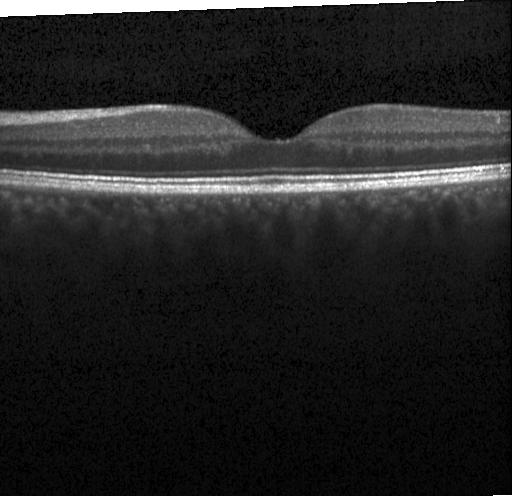

OCT line scan.
Macular OCT: no choroidal neovascularization, diabetic macular edema, or drusen.